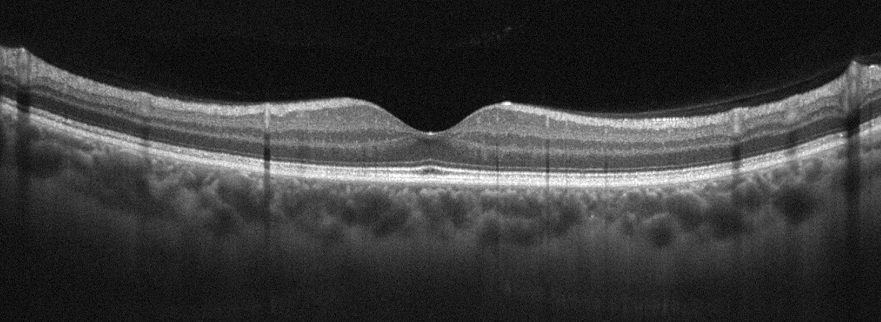
Macular OCT demonstrating no AMD, DME, ERM, RAO, RVO, or VID.